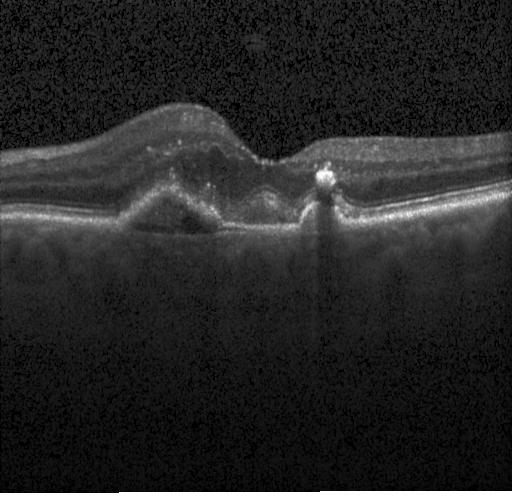
Macular scan; SD-OCT; OCT line scan; Heidelberg Spectralis. Impression: a choroidal neovascular membrane.